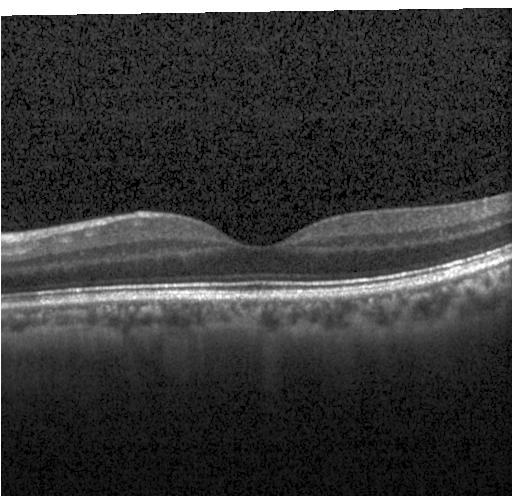

Retinal OCT cross-section showing neither choroidal neovascularization, diabetic macular edema, nor drusen.